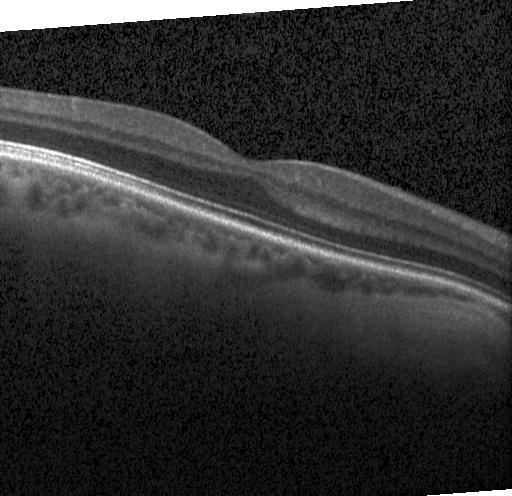
Macular scan. OCT line scan. SD-OCT. Heidelberg Spectralis OCT system — Finding: no choroidal neovascularization, no diabetic macular edema, and no drusen.